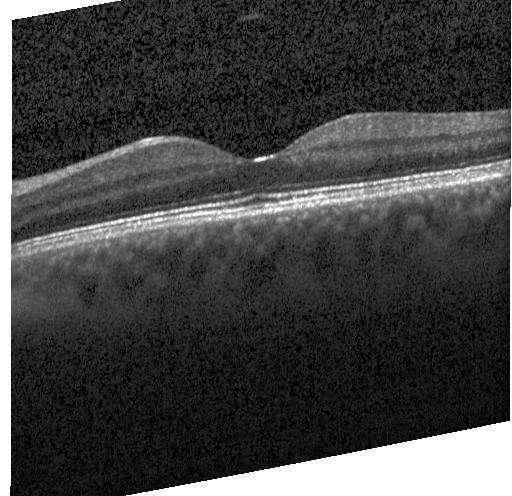
Fovea-centered; retinal OCT cross-section; SD-OCT; Heidelberg Spectralis OCT system. Impression: no CNV, DME, or drusen.